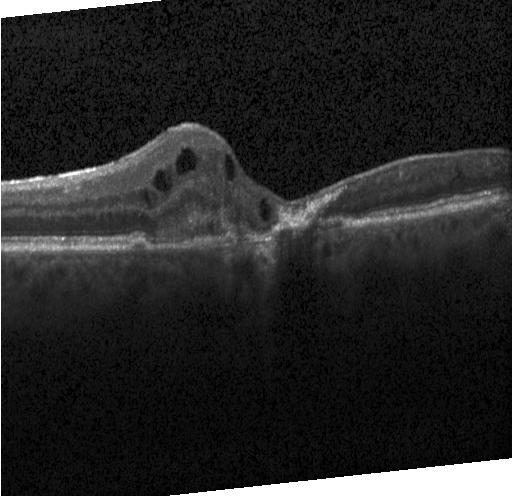

Spectral-domain OCT B-scan: choroidal neovascularization (CNV).